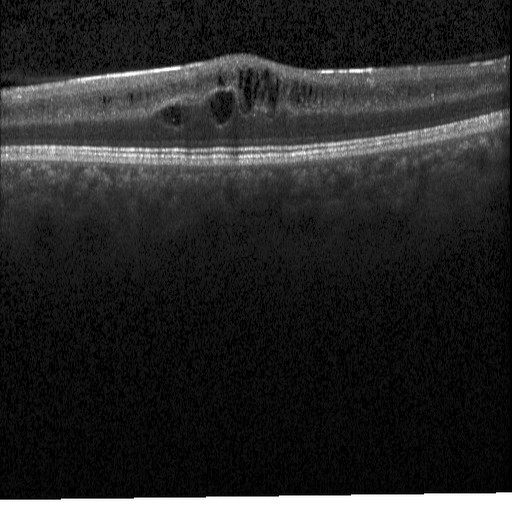 Impression: diabetic macular edema.